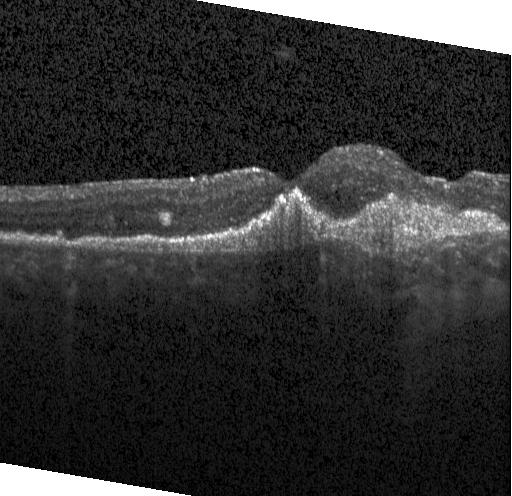
This B-scan demonstrates choroidal neovascularization (CNV).